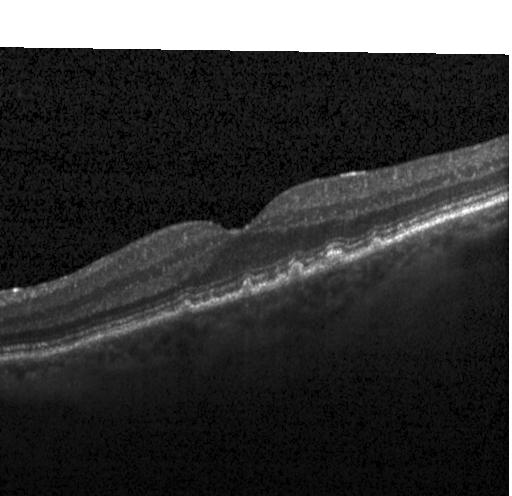 Horizontal scan through the fovea · spectral-domain optical coherence tomography · retinal OCT cross-section — Dx: sub-RPE drusenoid deposits.